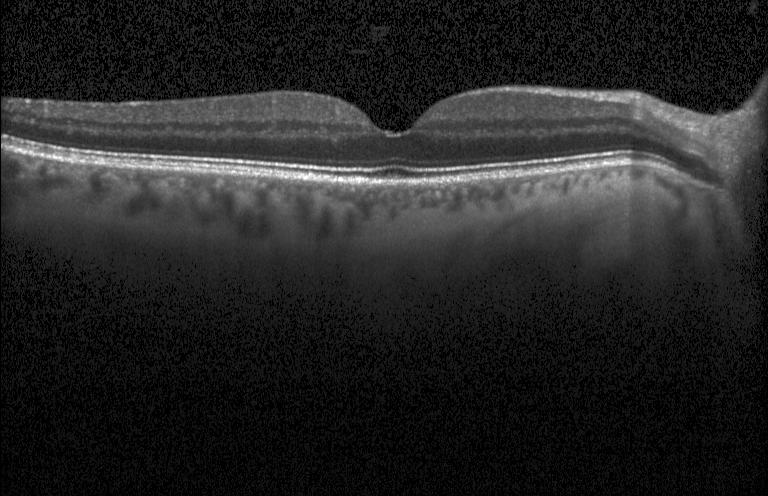 This B-scan demonstrates no choroidal neovascularization, no diabetic macular edema, and no drusen.